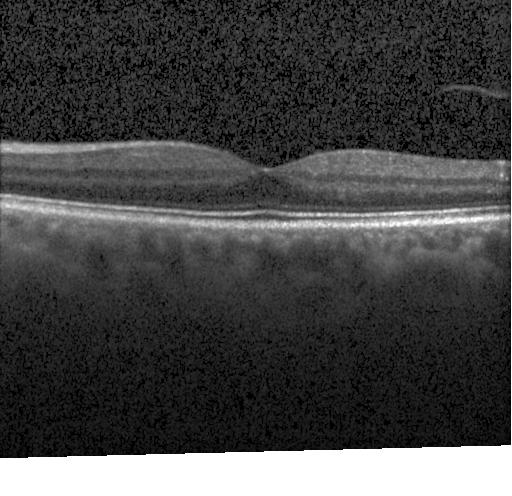

OCT B-scan. Through the macula.
Impression: neither CNV, DME, nor drusen.